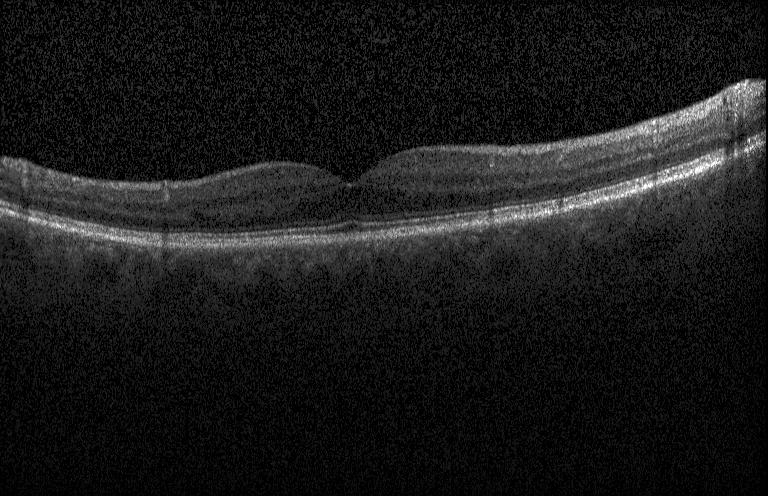
Macular OCT: no choroidal neovascularization, diabetic macular edema, or drusen.